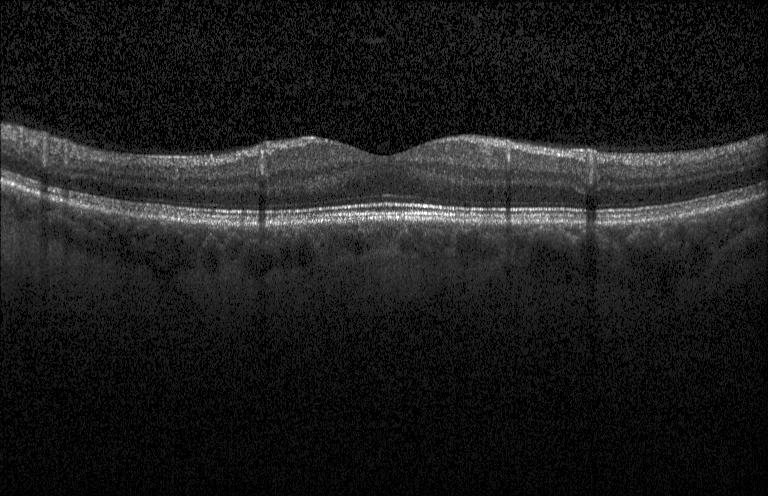

Spectral-domain OCT, retinal OCT cross-section
Finding: no evidence of choroidal neovascularization, diabetic macular edema, or drusen.